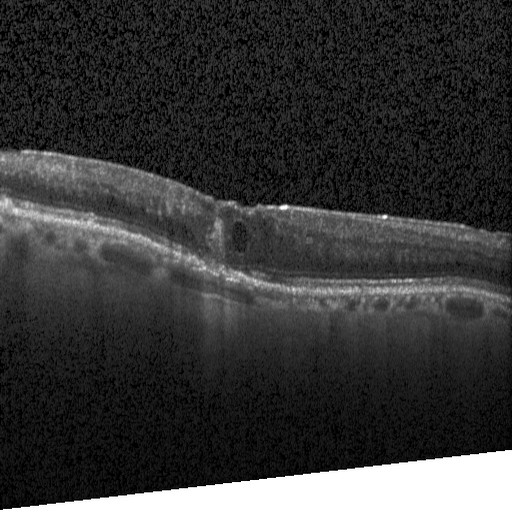
Diagnosis: DME.